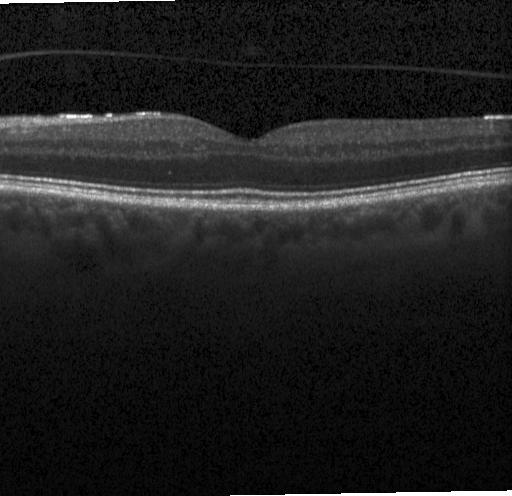

Finding: no CNV, DME, or drusen.